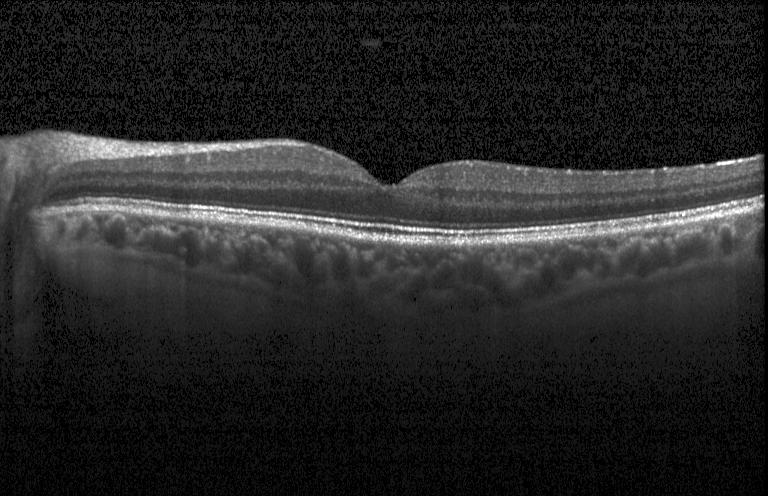 Dx: neither choroidal neovascularization, diabetic macular edema, nor drusen.